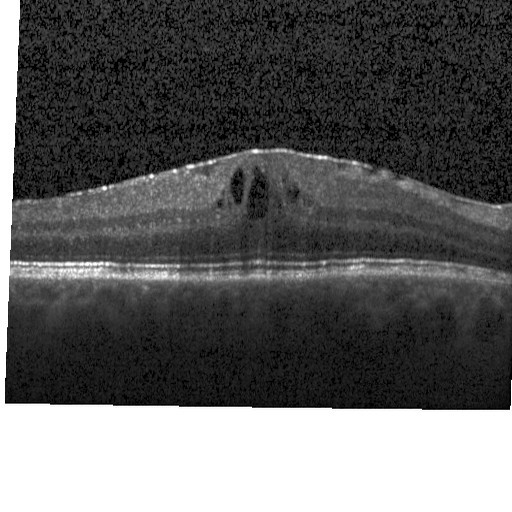
Impression: diabetic macular edema.